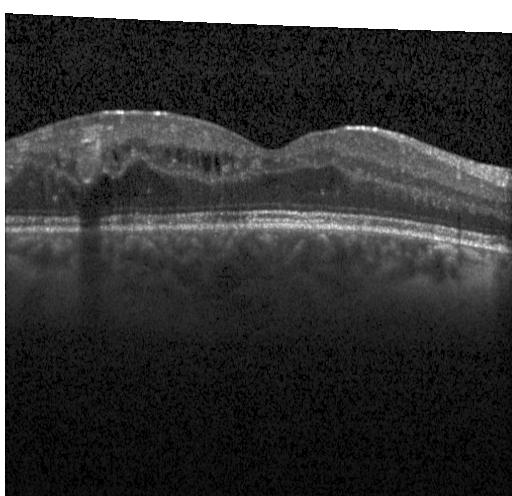 Optical coherence tomography scan.
Diagnosis: diabetic macular edema.